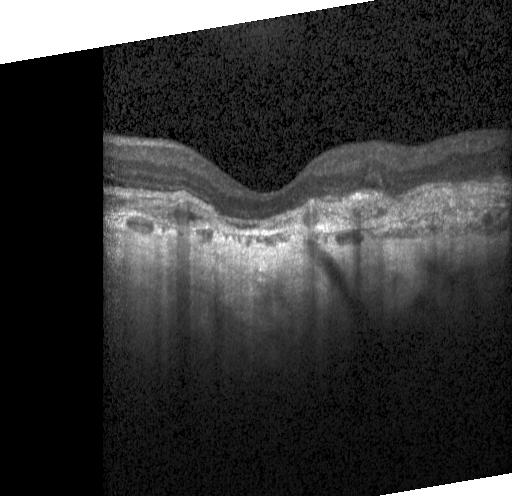
OCT finding: a choroidal neovascular membrane.